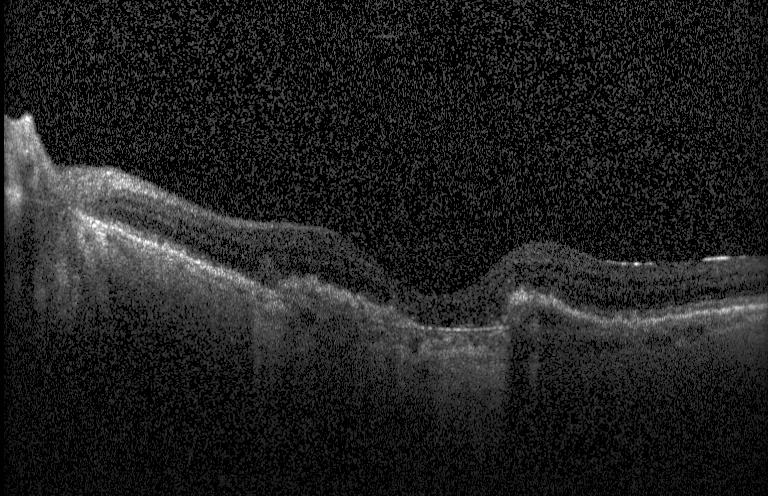
Finding: choroidal neovascularization.